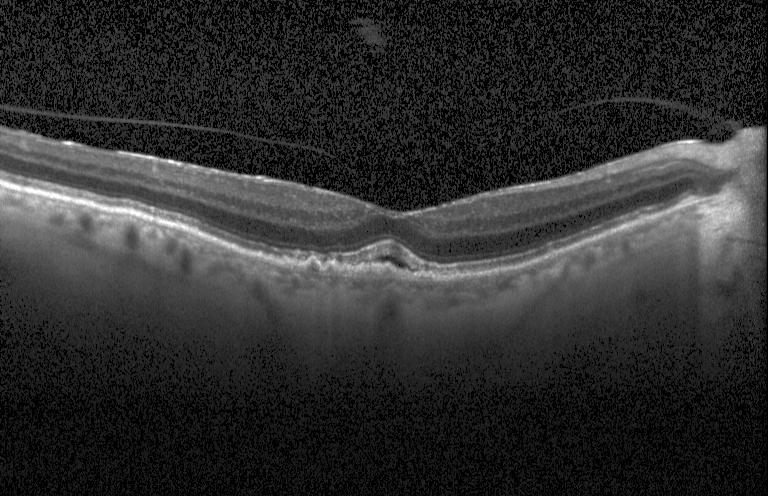 This B-scan demonstrates a choroidal neovascular membrane.